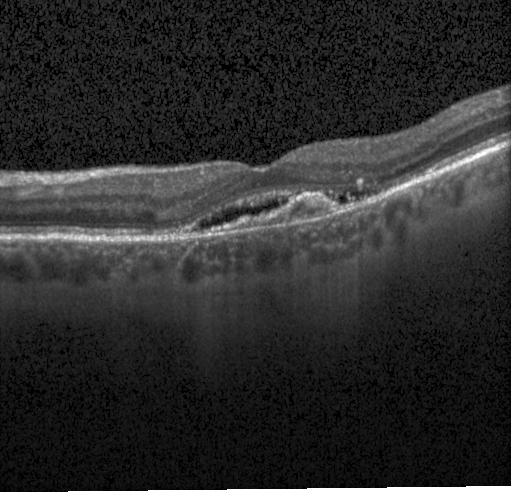
Instrument: Heidelberg Spectralis. Horizontal scan through the fovea. OCT B-scan. Impression: choroidal neovascularization.